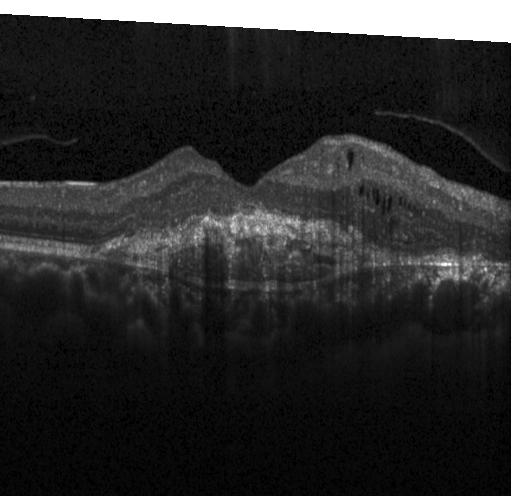 This B-scan demonstrates choroidal neovascularization.